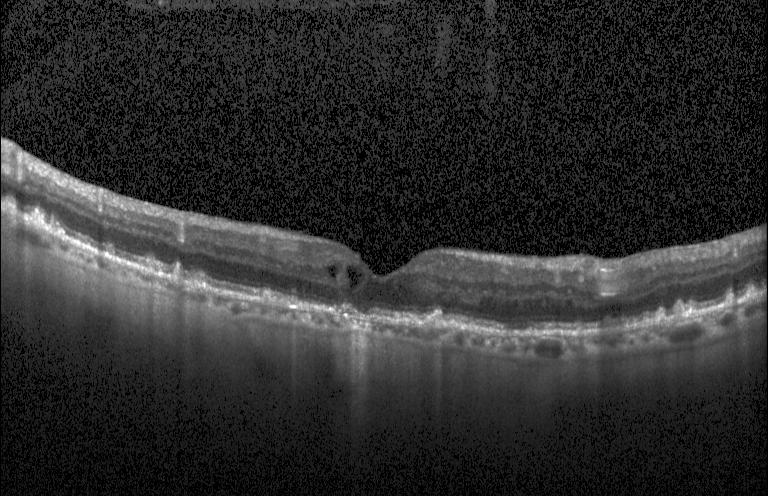

Retinal OCT B-scan — Choroidal neovascularization.